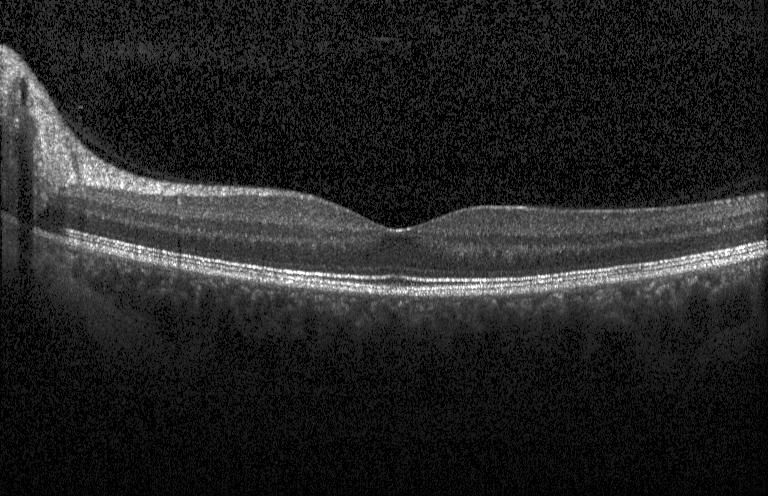

Centered on the fovea; optical coherence tomography scan — Assessment: no choroidal neovascularization, no diabetic macular edema, and no drusen.